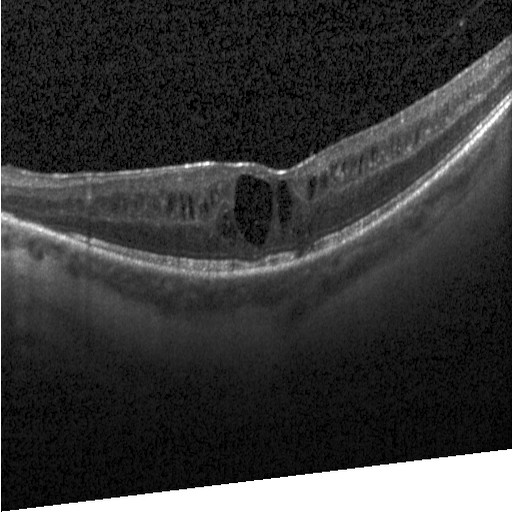

Fovea-centered, Heidelberg Spectralis OCT system, OCT B-scan. Assessment: diabetic macular edema.